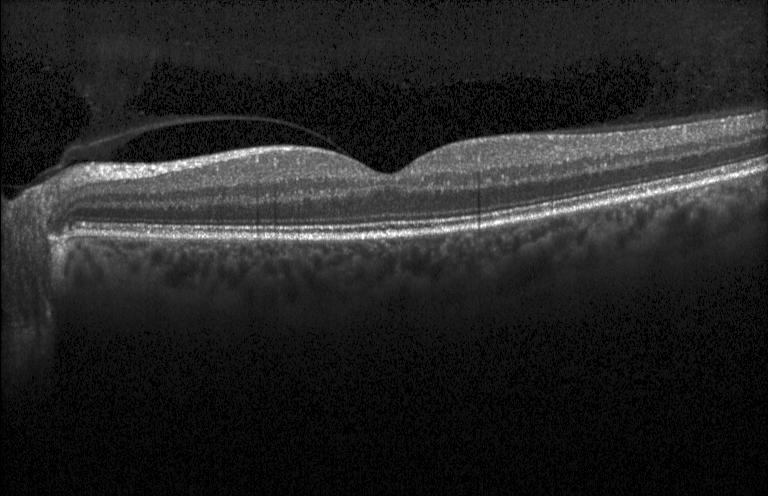 Optical coherence tomography B-scan; Heidelberg Spectralis; SD-OCT; through the macula — Assessment: no evidence of choroidal neovascularization, diabetic macular edema, or drusen.